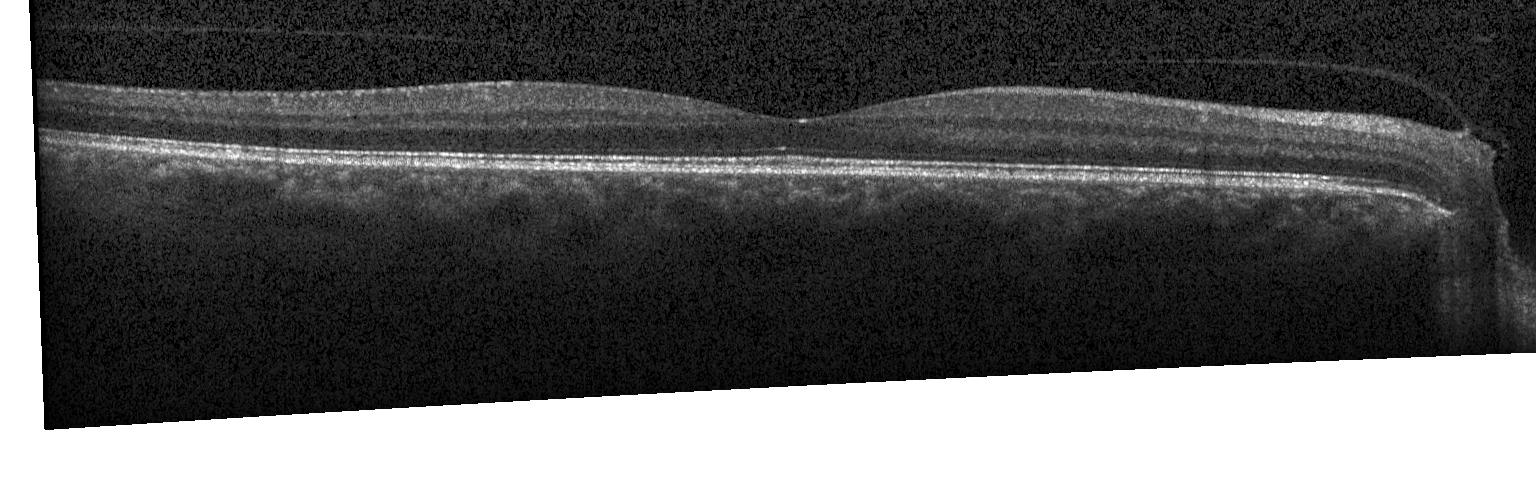

Horizontal scan through the fovea · SD-OCT · optical coherence tomography scan. Assessment: no evidence of CNV, DME, or drusen.